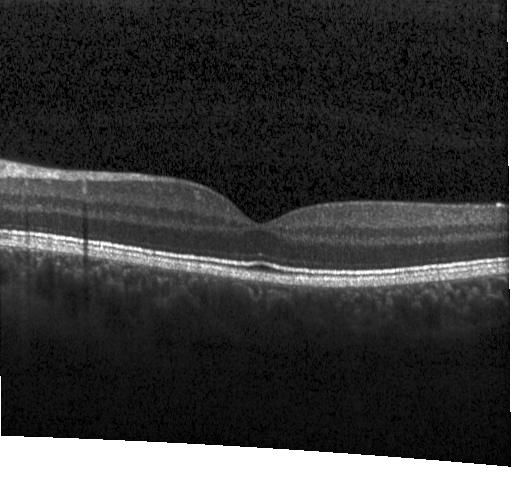 OCT scan showing no evidence of choroidal neovascularization, diabetic macular edema, or drusen.